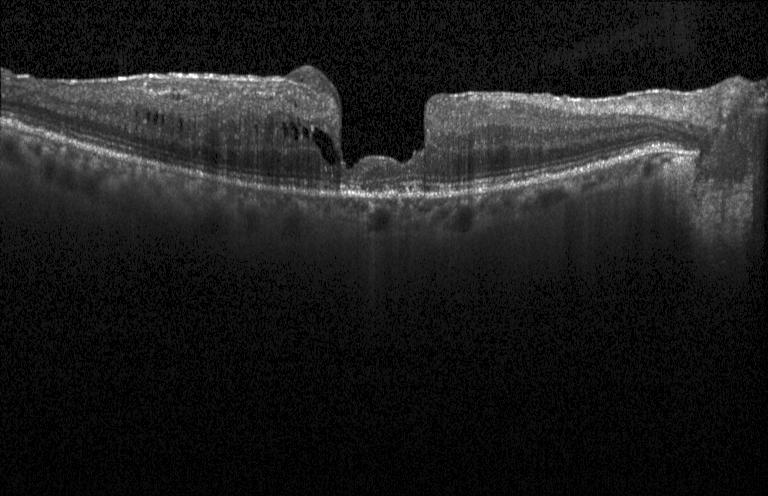
Horizontal scan through the fovea. OCT B-scan. Spectral-domain optical coherence tomography
Assessment: DME.